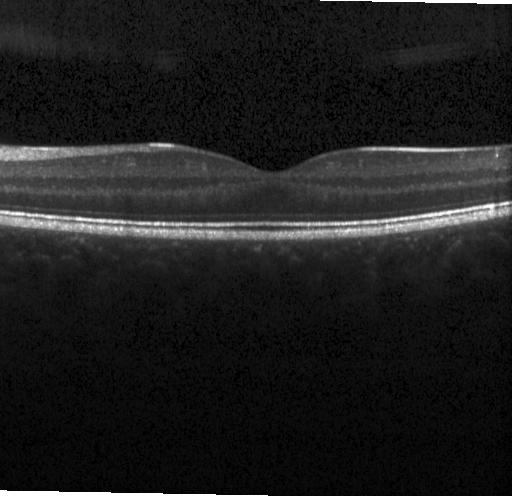
Macular scan. Heidelberg Spectralis. OCT line scan. SD-OCT. Impression: no evidence of CNV, DME, or drusen.